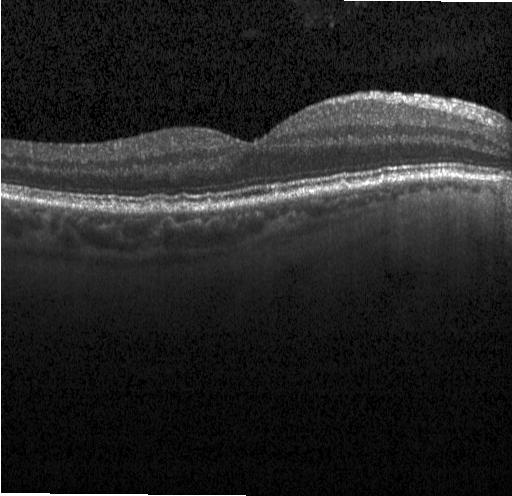

The scan shows sub-RPE drusenoid deposits.